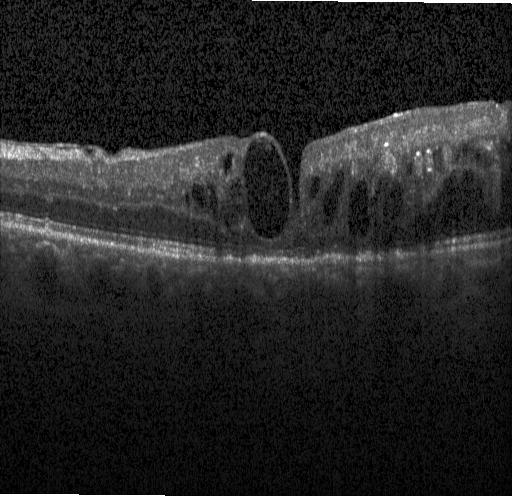

Finding: diabetic macular edema (DME).